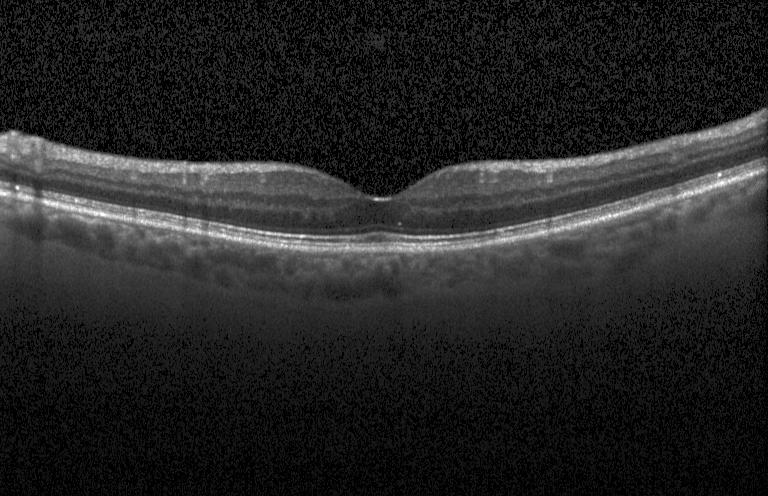 Impression: neither choroidal neovascularization, diabetic macular edema, nor drusen.